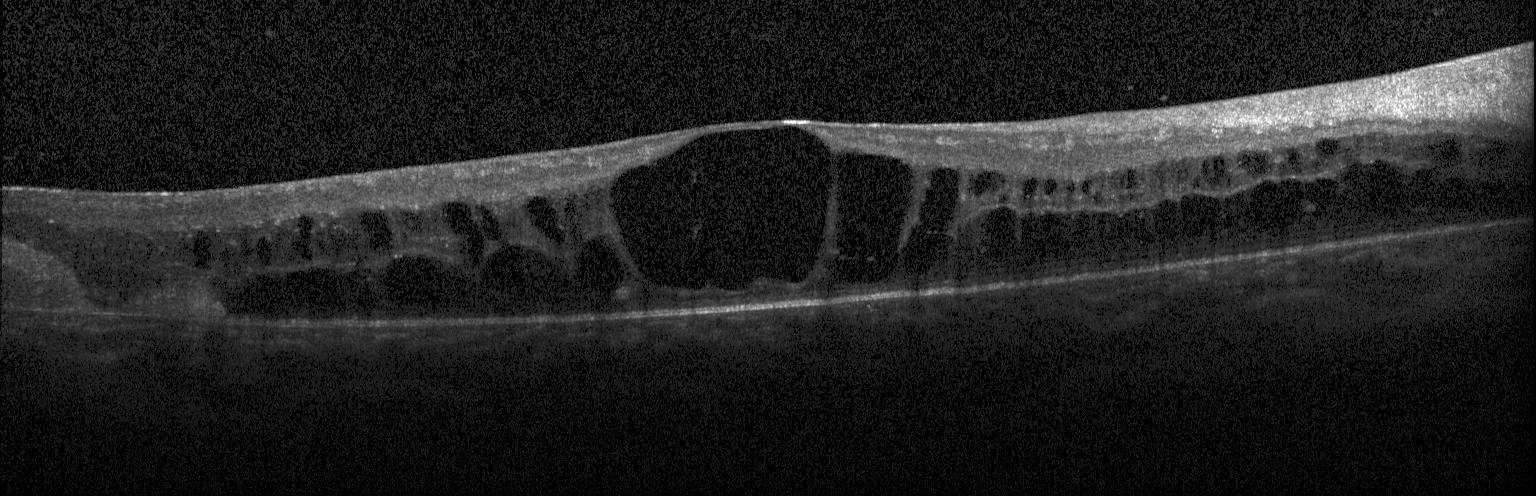

Retinal OCT B-scan · SD-OCT · Heidelberg Spectralis · through the macula. The scan shows diabetic macular edema.